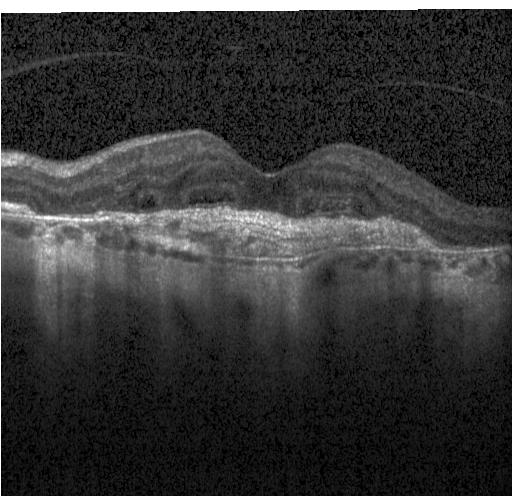

Optical coherence tomography B-scan.
Dx: a choroidal neovascular membrane.